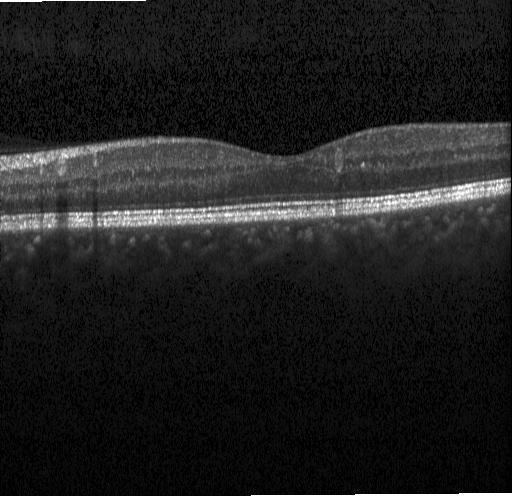 Acquired on a Heidelberg Spectralis; centered on the fovea; spectral-domain optical coherence tomography; optical coherence tomography B-scan. Assessment: no evidence of choroidal neovascularization, diabetic macular edema, or drusen.